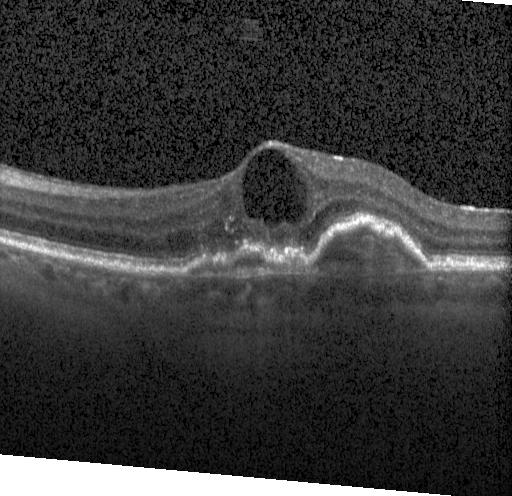
Through the macula. Optical coherence tomography B-scan. Spectral-domain OCT. This B-scan demonstrates a choroidal neovascular membrane.